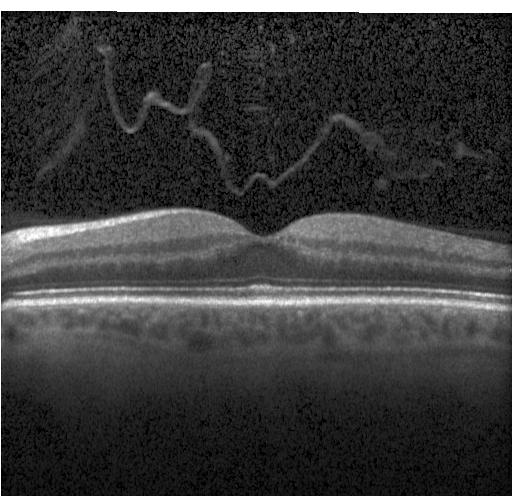
Optical coherence tomography B-scan · centered on the fovea — No evidence of CNV, DME, or drusen.